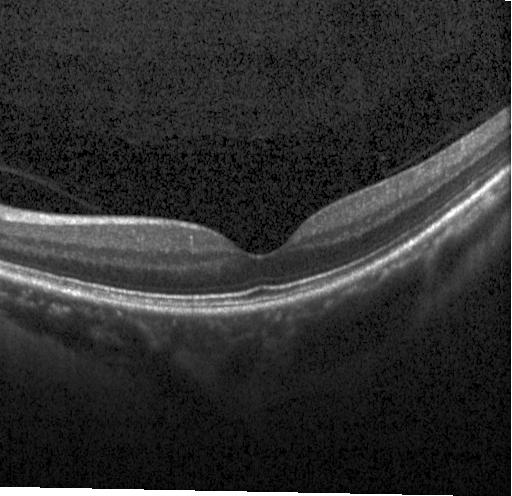 Diagnosis: no choroidal neovascularization, no diabetic macular edema, and no drusen.